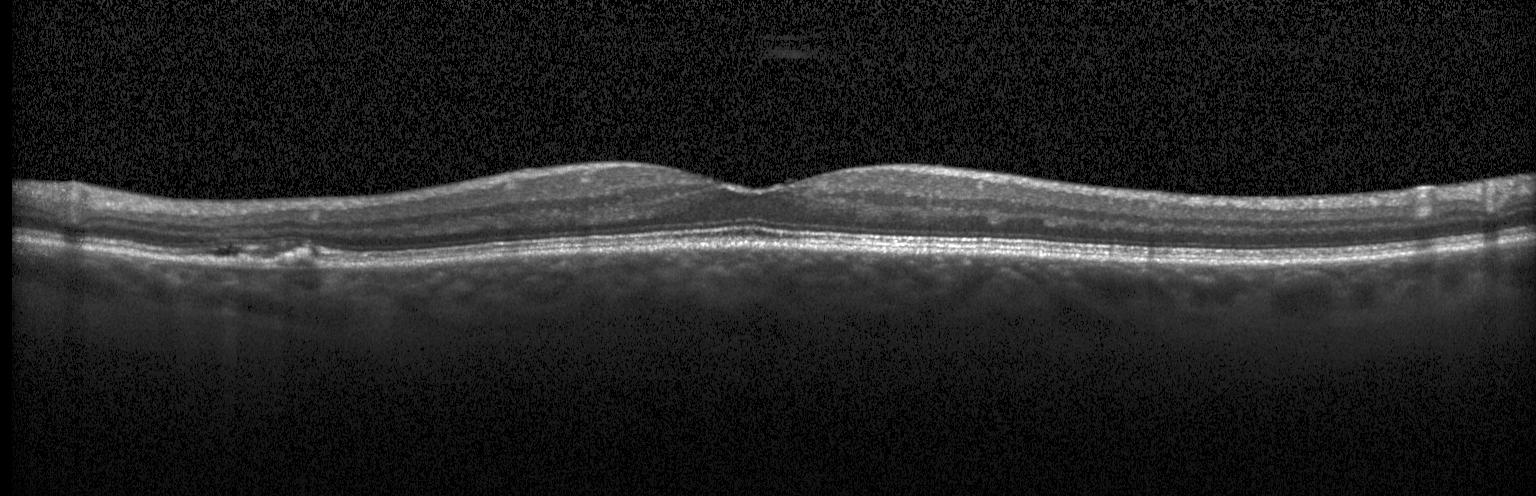 Horizontal scan through the fovea · retinal OCT B-scan.
Dx: choroidal neovascularization.